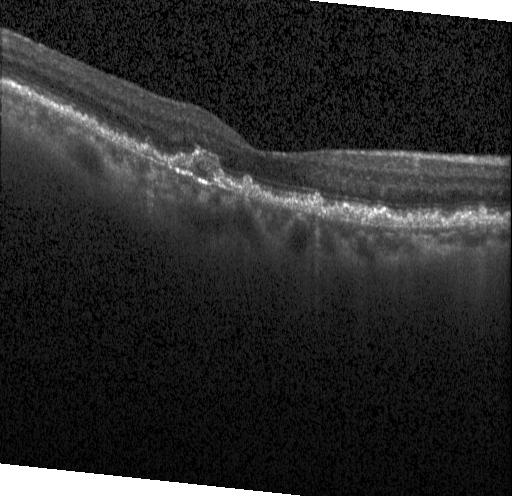
OCT scan showing a choroidal neovascular membrane.